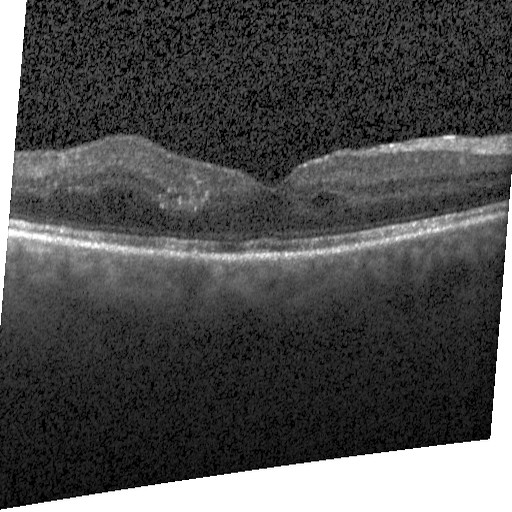 OCT line scan. Assessment: DME.